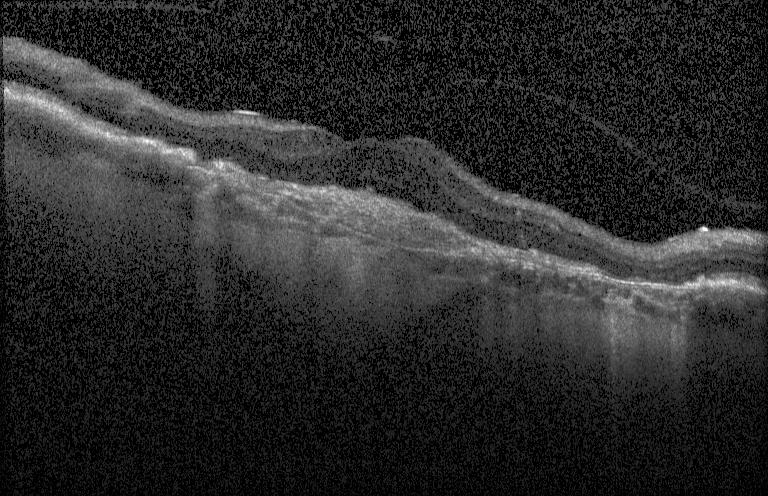 Optical coherence tomography B-scan
Diagnosis: choroidal neovascularization (CNV).